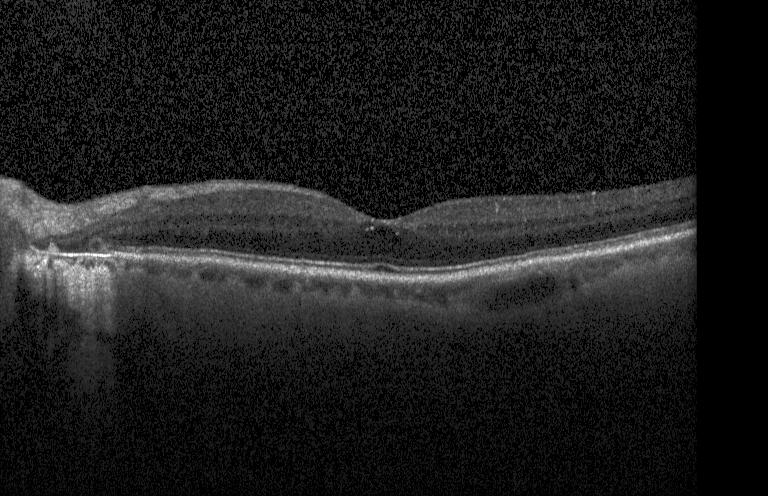 OCT line scan · horizontal scan through the fovea
Assessment: no evidence of CNV, DME, or drusen.